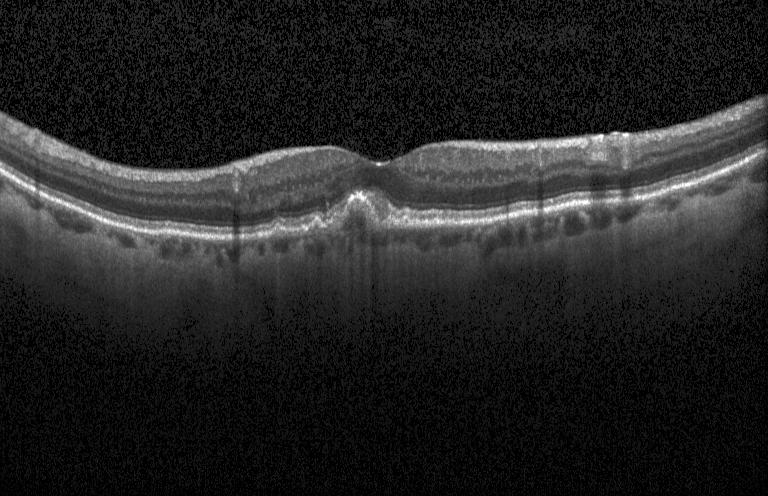

Optical coherence tomography B-scan — Diagnosis: multiple drusen.